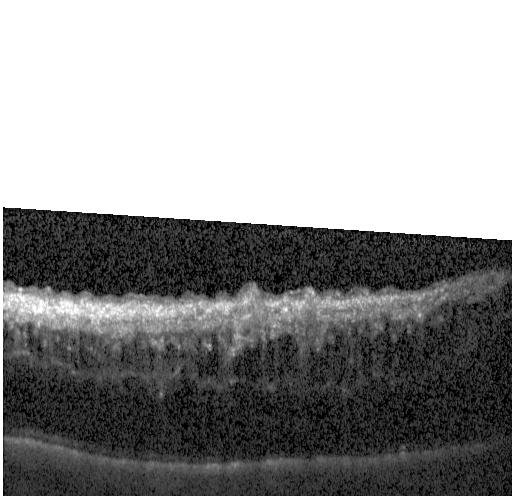
Through the macula · retinal OCT B-scan
The scan shows diabetic macular edema.